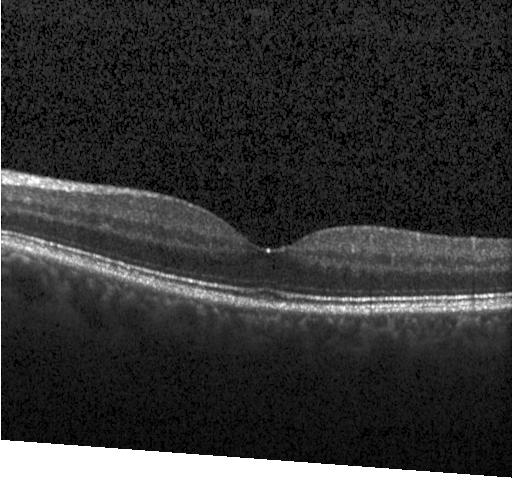
Optical coherence tomography scan.
Finding: neither choroidal neovascularization, diabetic macular edema, nor drusen.